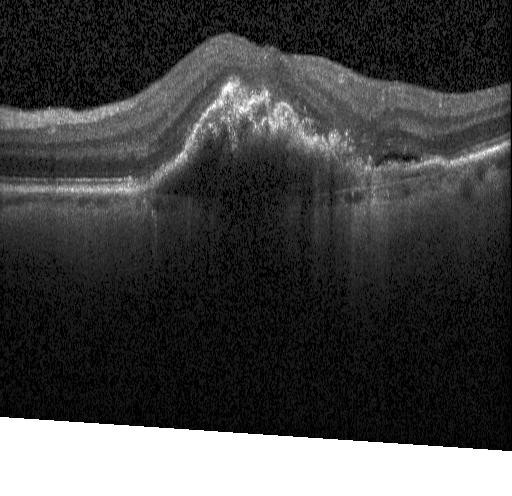
Through the macula, spectral-domain OCT, OCT line scan. This B-scan demonstrates CNV.